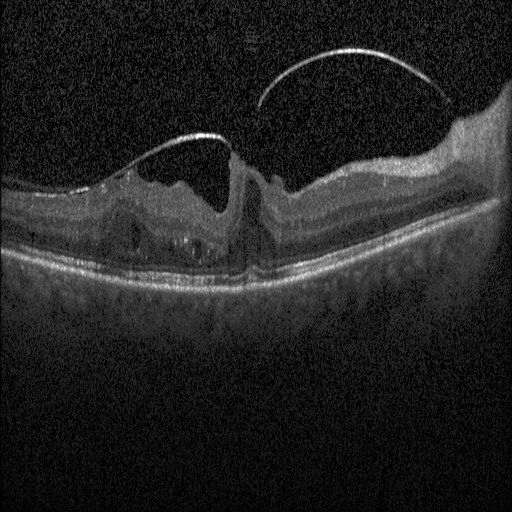 Optical coherence tomography scan, macular scan — Impression: diabetic macular edema.